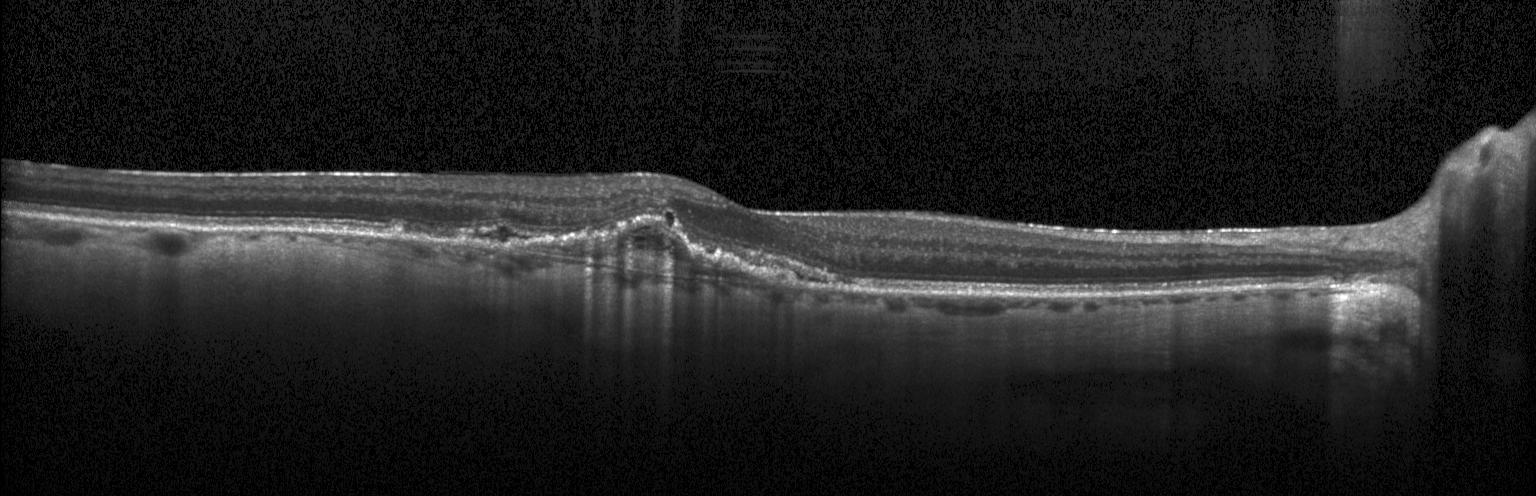

This B-scan demonstrates a choroidal neovascular membrane.